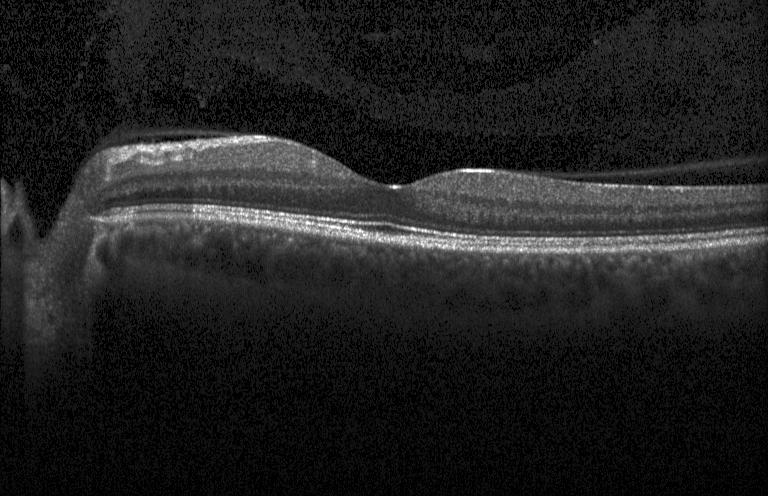

Diagnosis: no choroidal neovascularization, diabetic macular edema, or drusen.